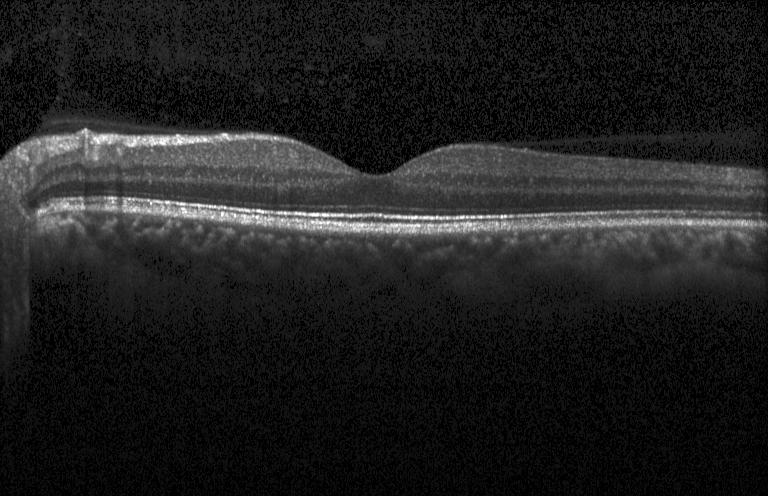

Diagnosis: no choroidal neovascularization, no diabetic macular edema, and no drusen.